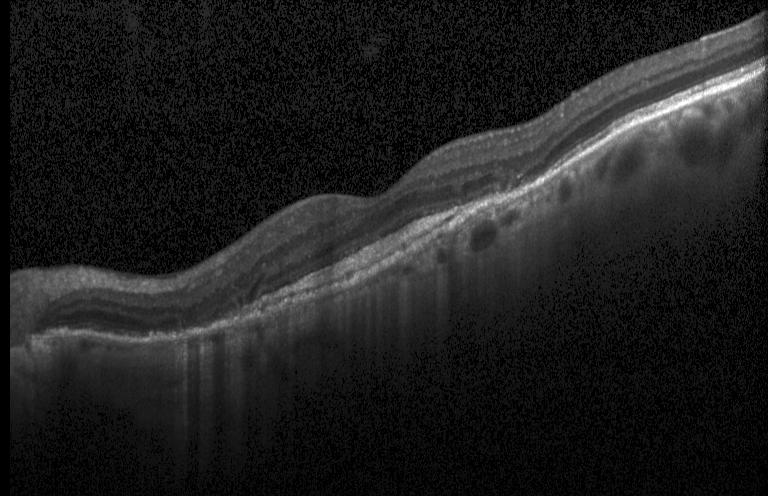

OCT finding: choroidal neovascularization (CNV).